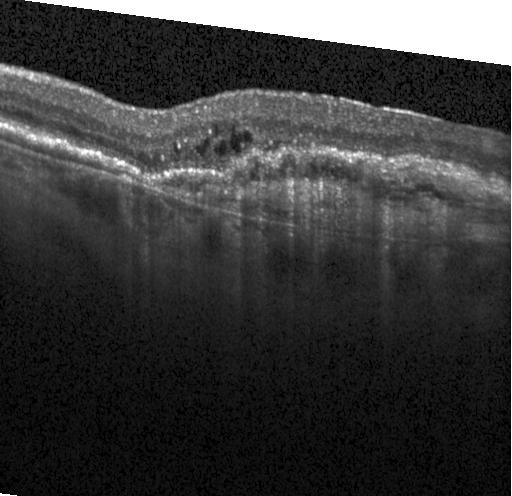

SD-OCT · centered on the fovea · optical coherence tomography scan · Heidelberg Spectralis OCT system. This B-scan demonstrates a choroidal neovascular membrane.